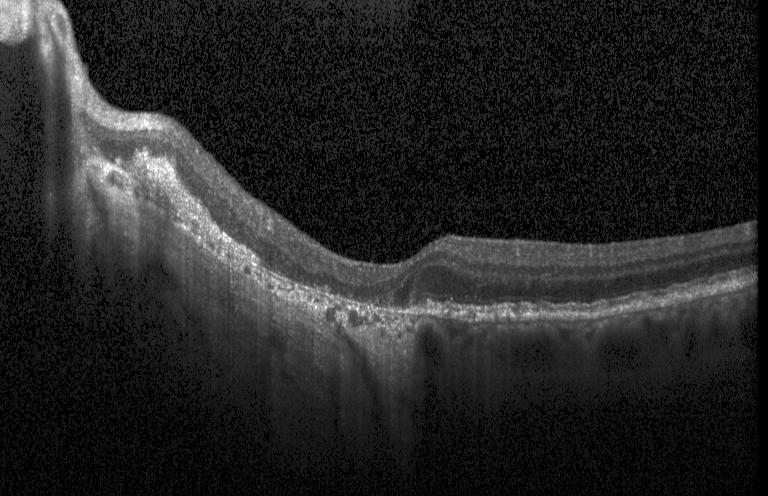 Impression: CNV.